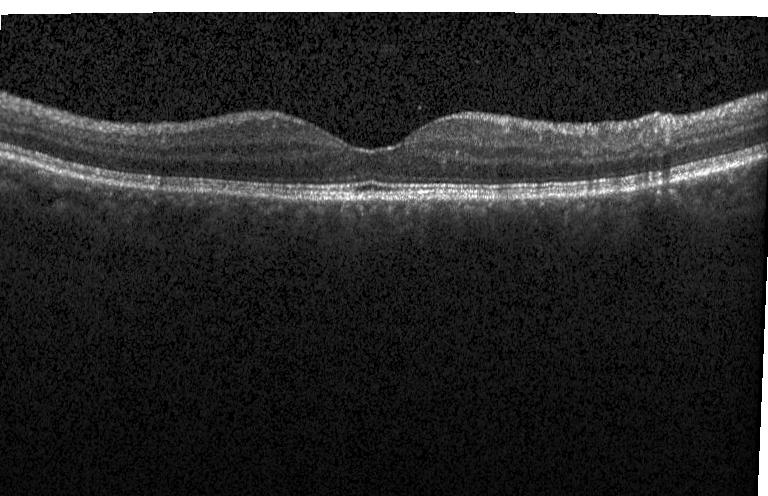

Macular OCT demonstrating no choroidal neovascularization, no diabetic macular edema, and no drusen.